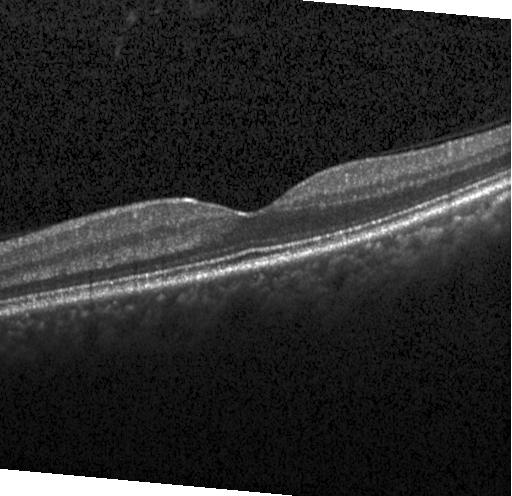 Retinal OCT cross-section. No choroidal neovascularization, no diabetic macular edema, and no drusen.